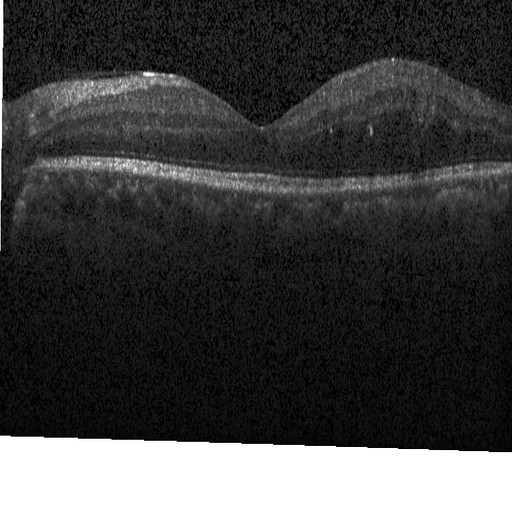

Spectral-domain OCT, instrument: Heidelberg Spectralis, retinal OCT B-scan
OCT finding: DME.